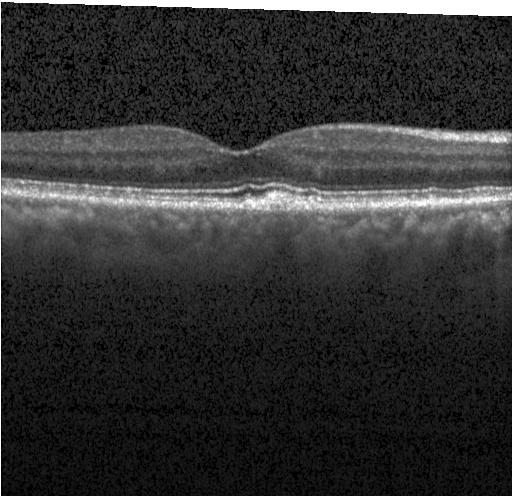 OCT B-scan — Dx: sub-RPE drusenoid deposits.